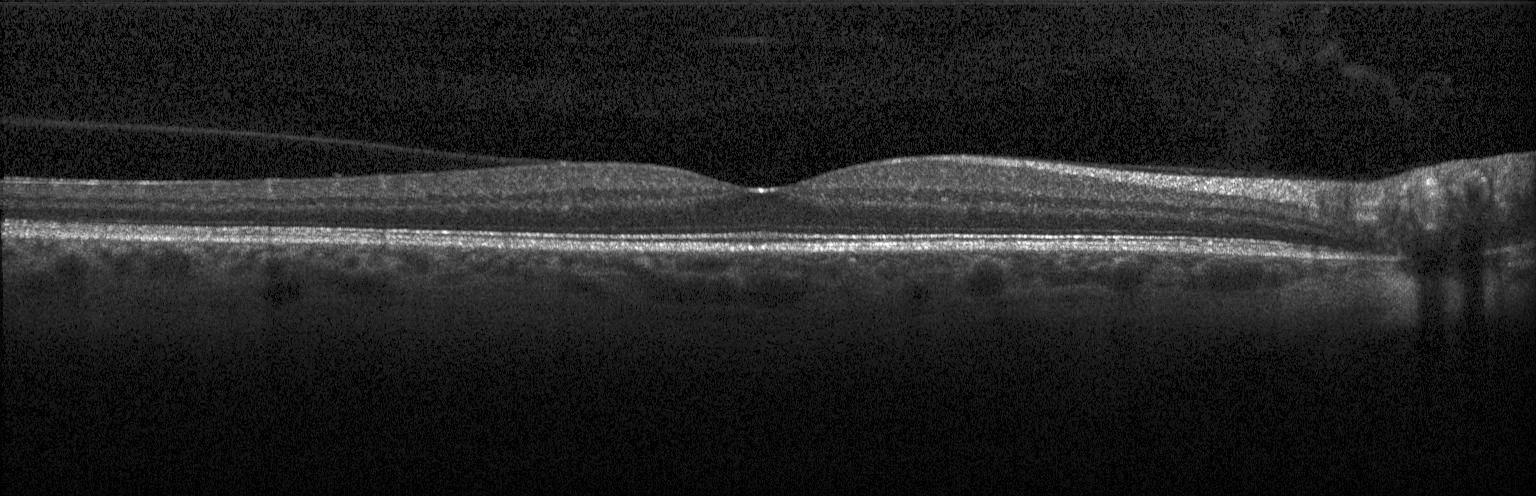
OCT line scan.
OCT finding: no choroidal neovascularization, diabetic macular edema, or drusen.